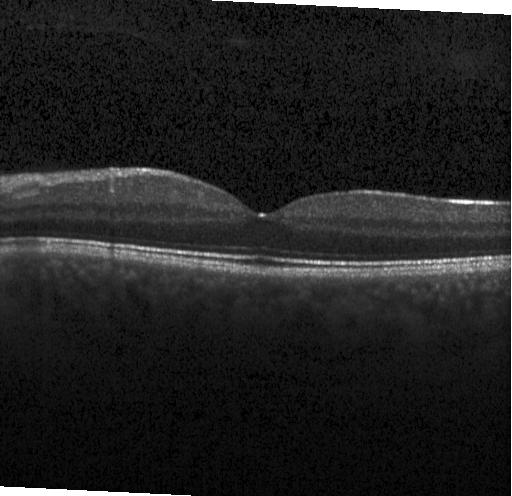 OCT B-scan; instrument: Heidelberg Spectralis; fovea-centered
Impression: no choroidal neovascularization, no diabetic macular edema, and no drusen.